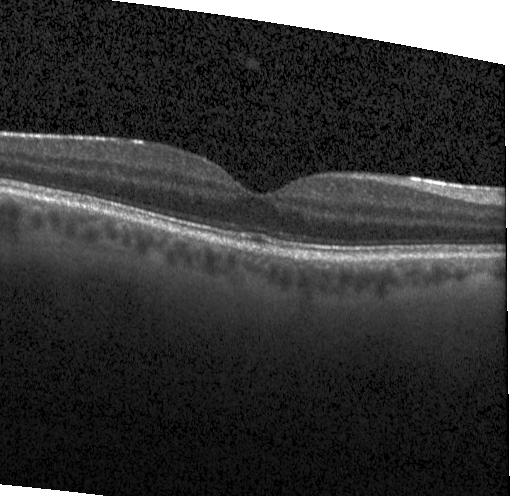 Finding: no choroidal neovascularization, diabetic macular edema, or drusen.